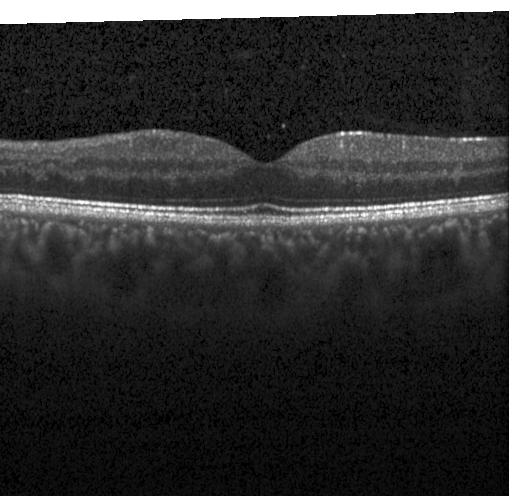
Assessment: no choroidal neovascularization, no diabetic macular edema, and no drusen.